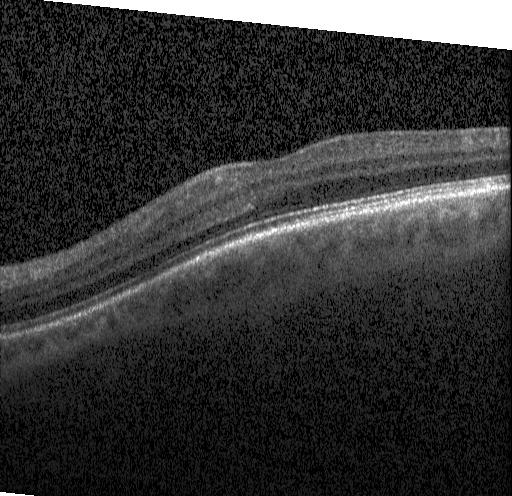 Optical coherence tomography B-scan. No choroidal neovascularization, diabetic macular edema, or drusen.